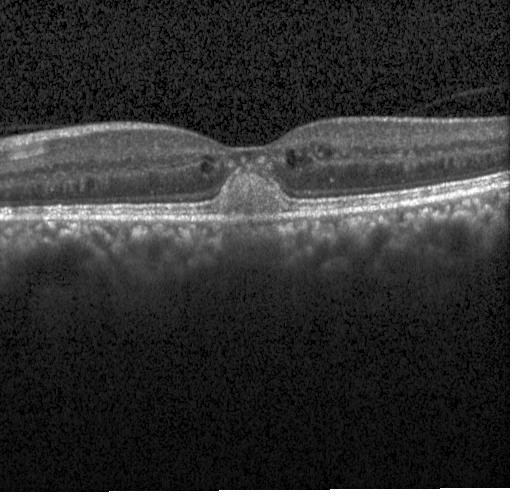
Impression: choroidal neovascularization (CNV).